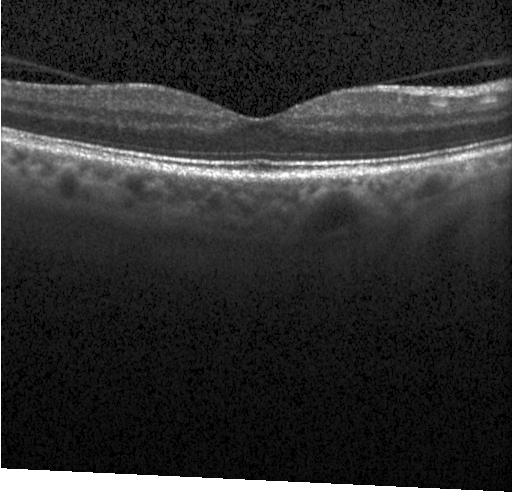
Heidelberg Spectralis; spectral-domain OCT; optical coherence tomography B-scan; horizontal scan through the fovea — The scan shows no choroidal neovascularization, diabetic macular edema, or drusen.